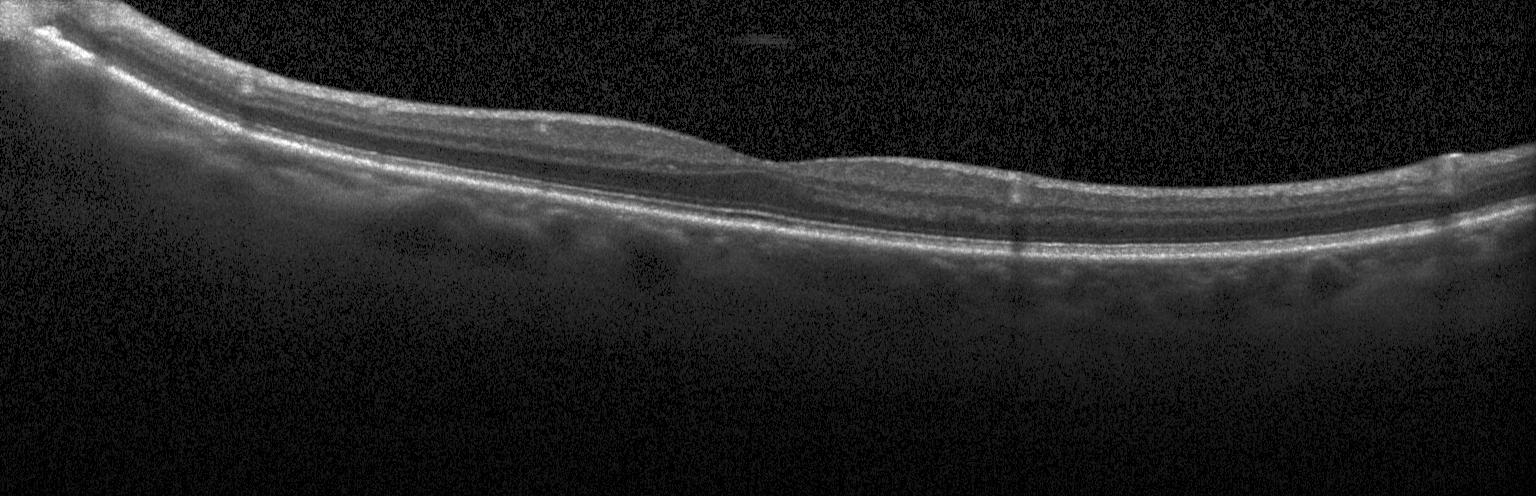
Optical coherence tomography B-scan.
Dx: no CNV, DME, or drusen.